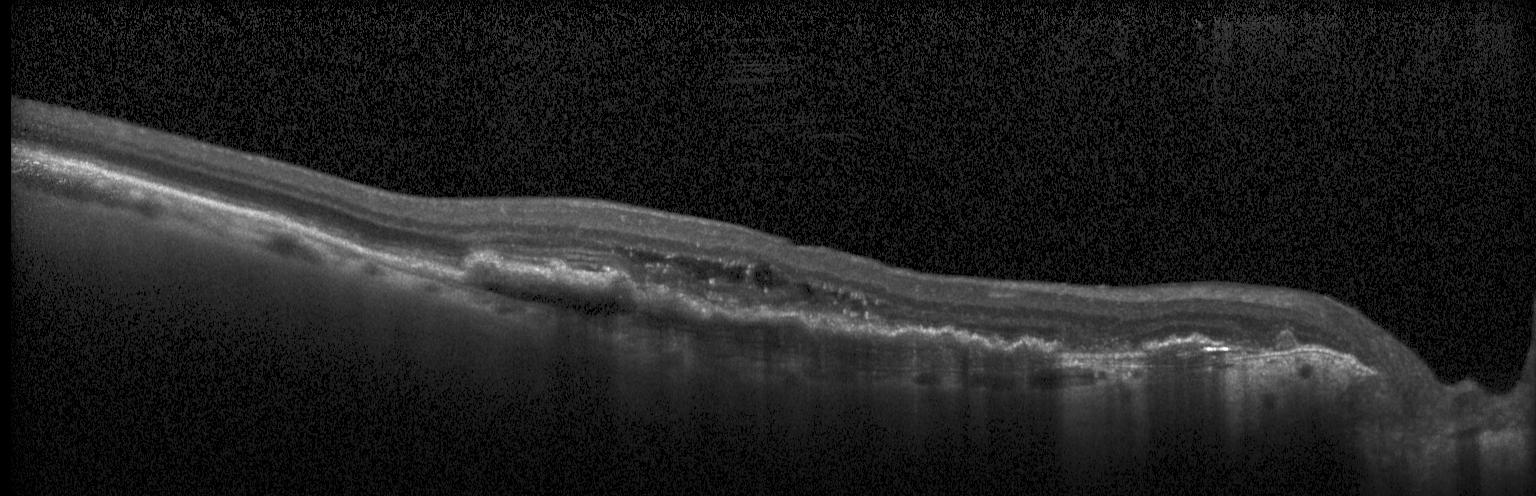 Finding: a choroidal neovascular membrane.